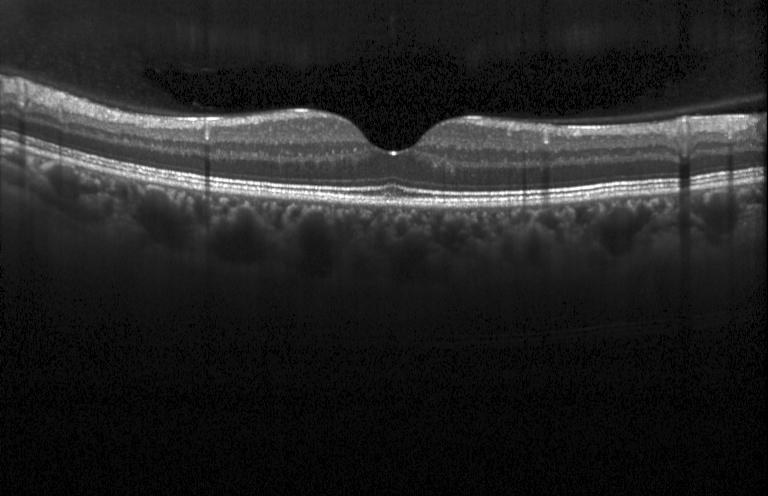
Optical coherence tomography scan. Through the macula. The scan shows no choroidal neovascularization, no diabetic macular edema, and no drusen.